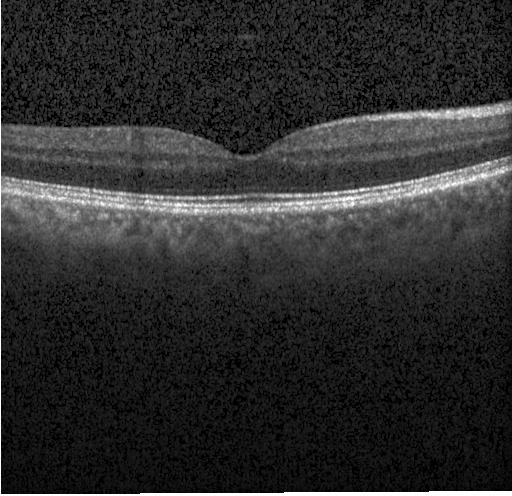 OCT B-scan — This B-scan demonstrates neither choroidal neovascularization, diabetic macular edema, nor drusen.